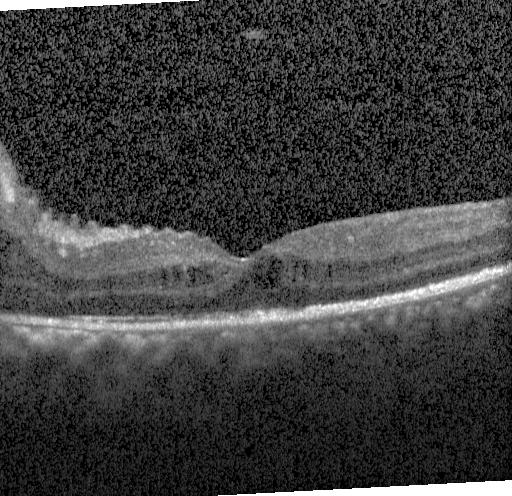

OCT B-scan
Assessment: diabetic macular edema (DME).